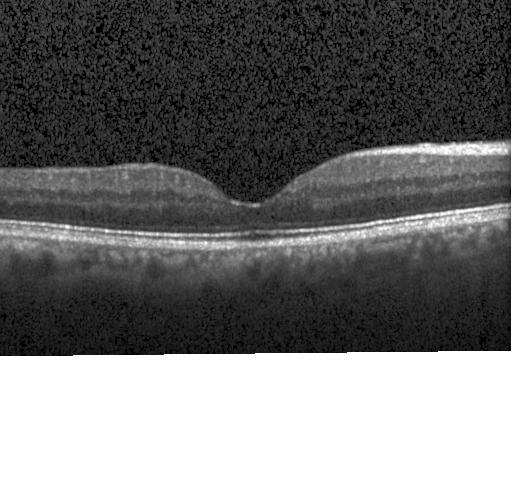

Diagnosis: no CNV, DME, or drusen.